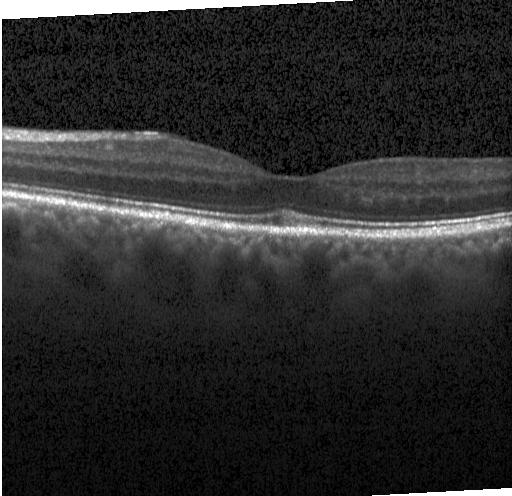
Macular OCT: no CNV, DME, or drusen.